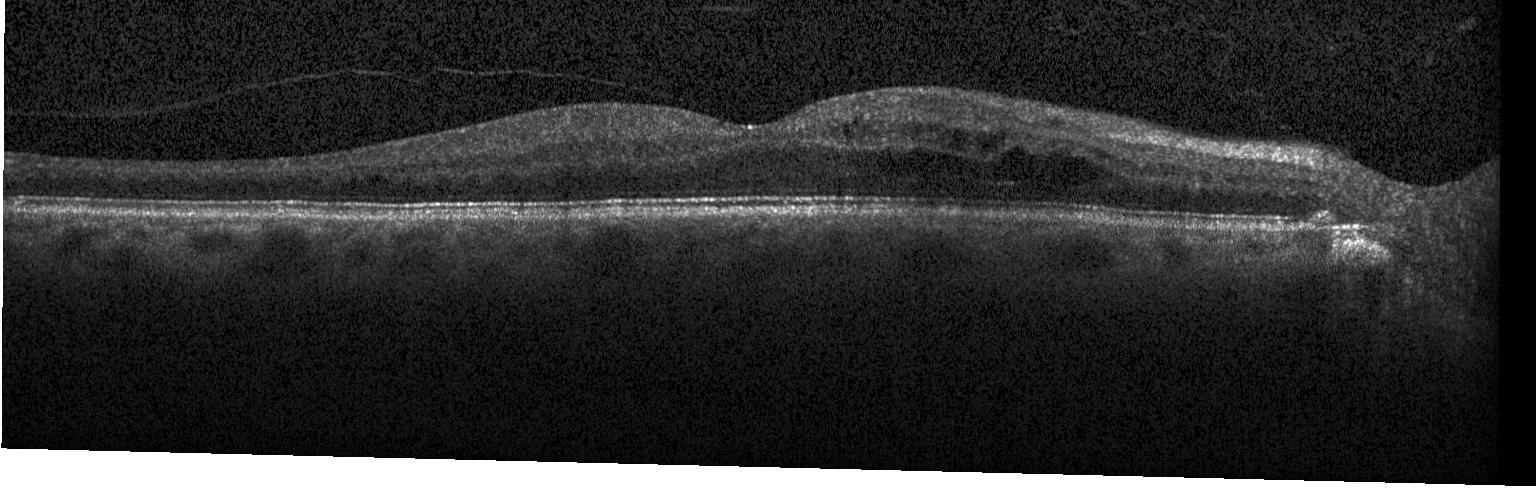 Retinal OCT cross-section showing diabetic macular edema.